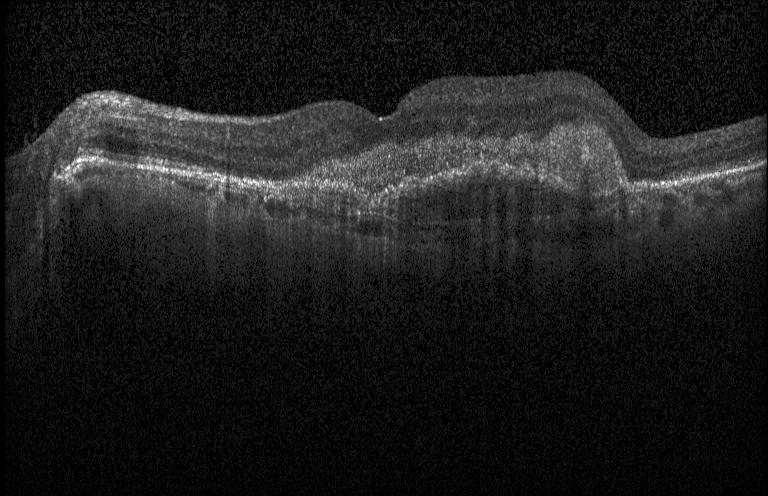
Retinal OCT cross-section. Centered on the fovea. SD-OCT
Impression: a choroidal neovascular membrane.